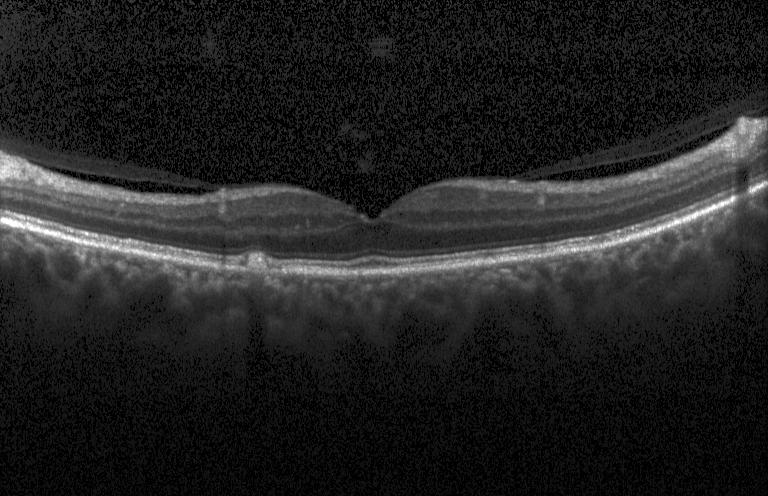 Spectral-domain OCT B-scan: multiple drusen.